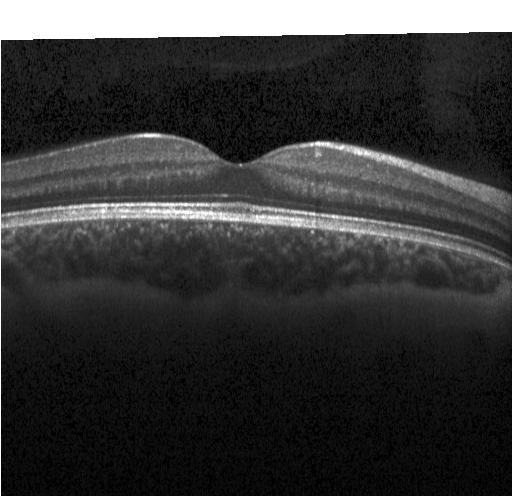 Diagnosis: no CNV, DME, or drusen.